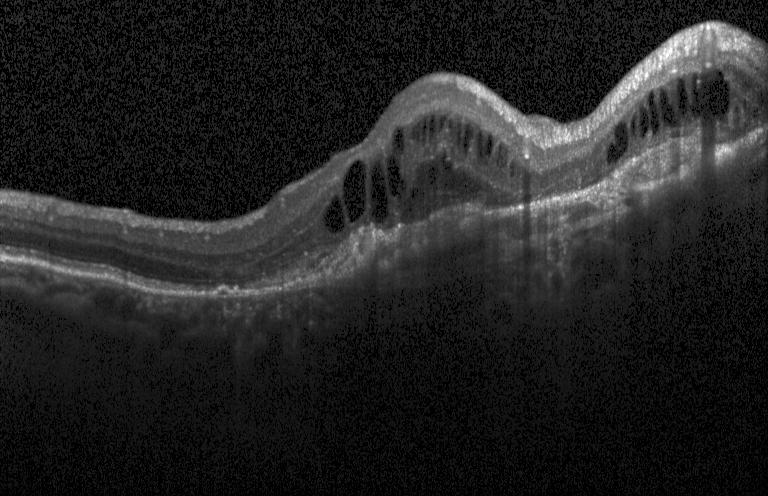
Diagnosis: a choroidal neovascular membrane.